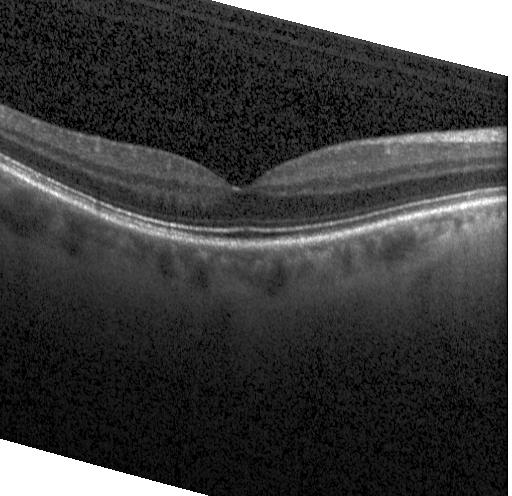 Spectral-domain OCT; OCT B-scan.
Impression: no CNV, DME, or drusen.